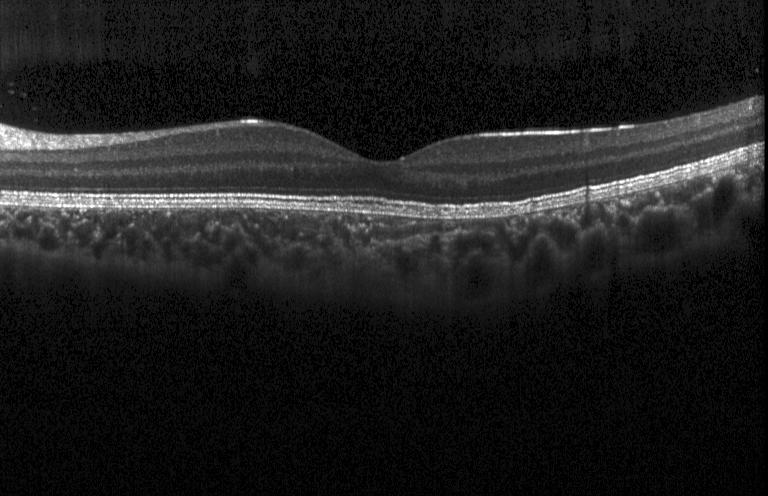
Spectral-domain OCT, macular scan, optical coherence tomography B-scan. Neither CNV, DME, nor drusen.